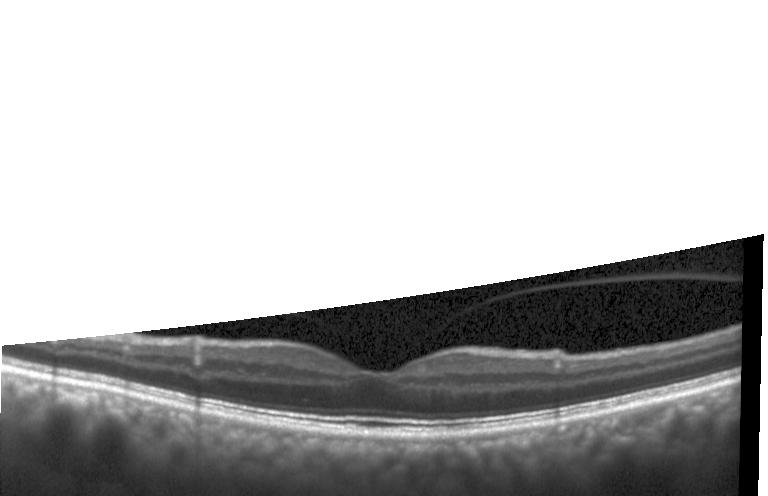
OCT finding: no choroidal neovascularization, no diabetic macular edema, and no drusen.